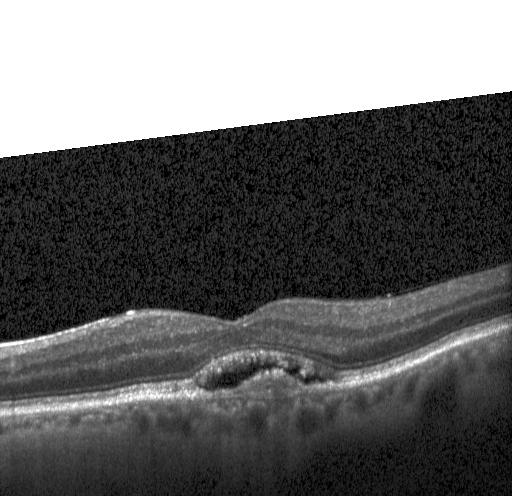 Optical coherence tomography B-scan. The scan shows CNV.